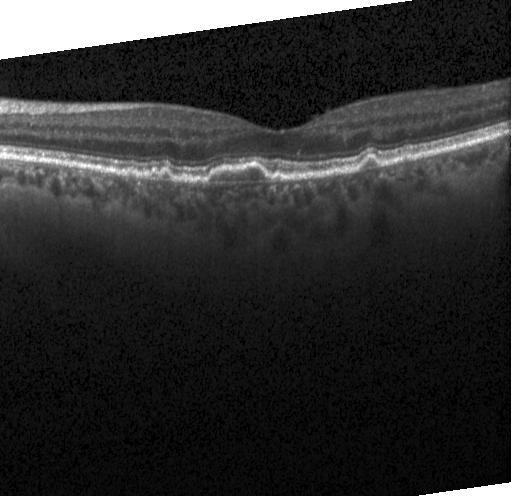

Heidelberg Spectralis OCT system; retinal OCT cross-section; horizontal scan through the fovea. The scan shows sub-RPE drusenoid deposits.